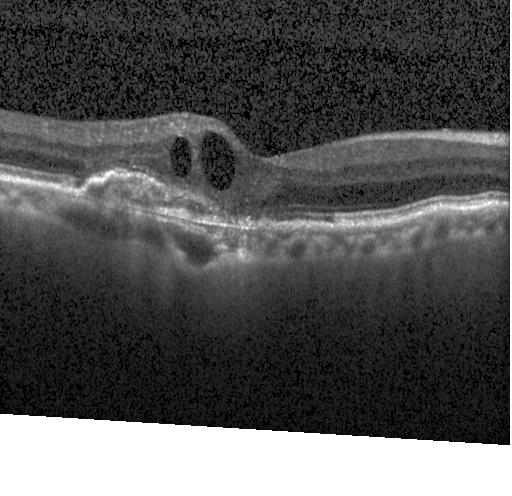 OCT scan showing a choroidal neovascular membrane.